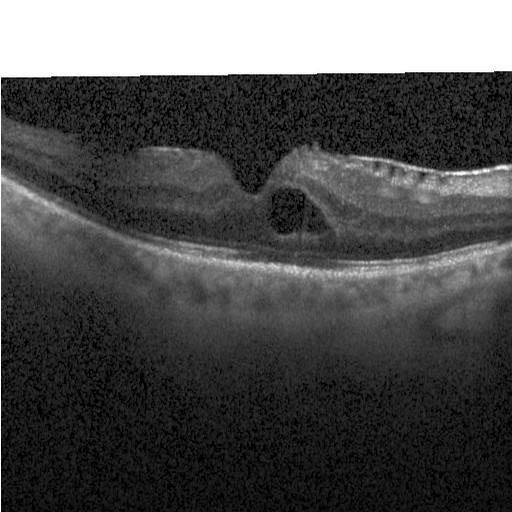
Fovea-centered, retinal OCT cross-section
Dx: diabetic macular edema (DME).